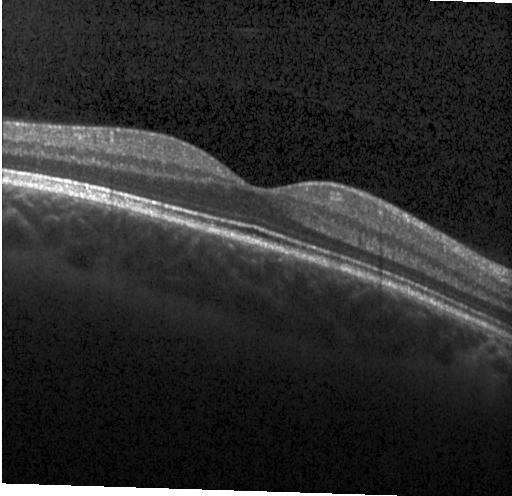 Optical coherence tomography B-scan. Heidelberg Spectralis
No CNV, DME, or drusen.